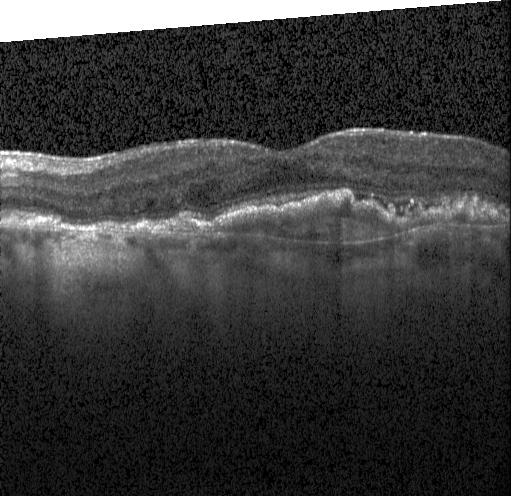
Macular OCT demonstrating choroidal neovascularization (CNV).